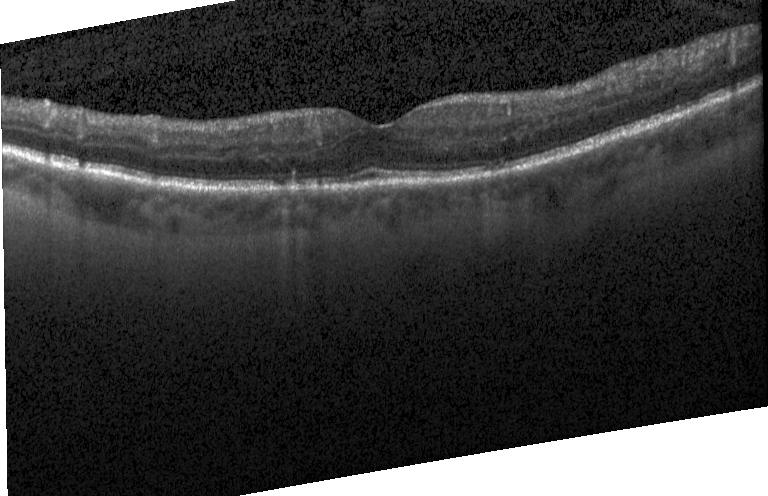
Optical coherence tomography scan, horizontal scan through the fovea
This B-scan demonstrates diabetic macular edema.